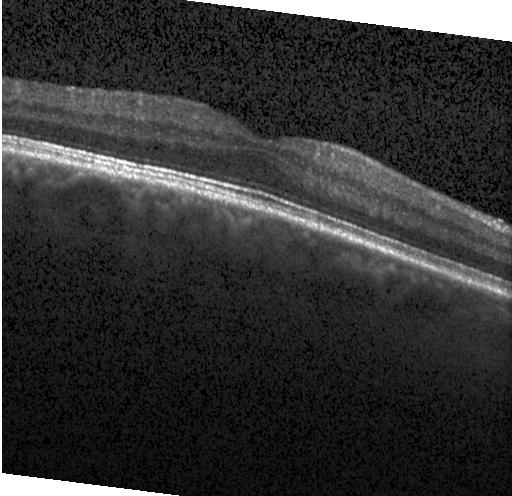 Finding: no choroidal neovascularization, diabetic macular edema, or drusen.